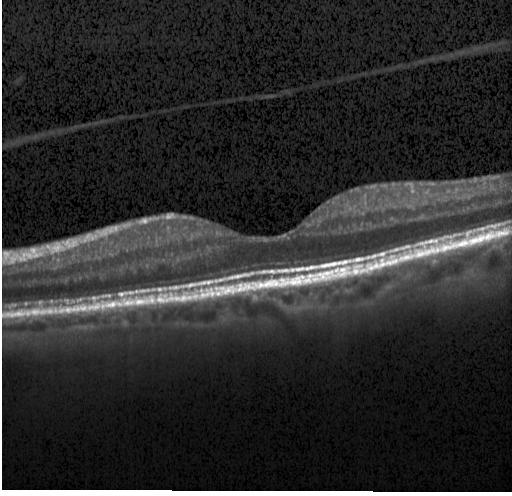
Retinal OCT B-scan, through the macula, spectral-domain OCT.
Finding: no evidence of choroidal neovascularization, diabetic macular edema, or drusen.